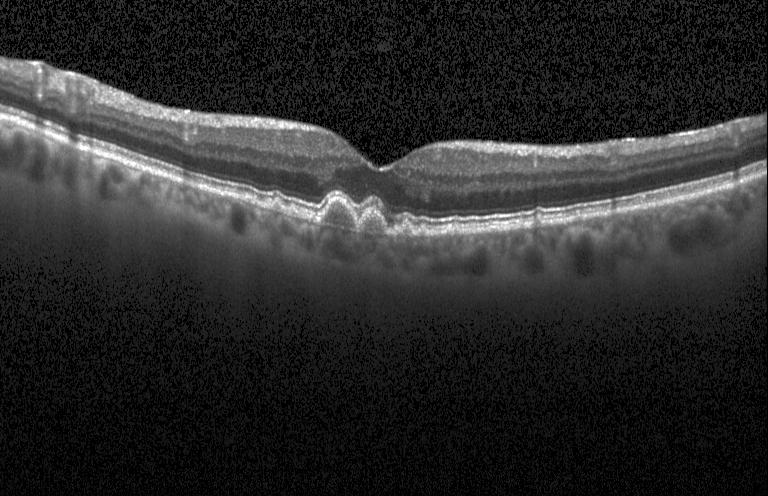
Retinal OCT B-scan.
Sub-RPE drusenoid deposits.